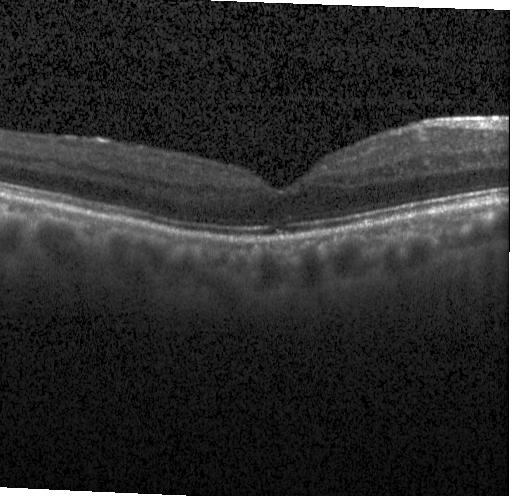

Finding: no choroidal neovascularization, no diabetic macular edema, and no drusen.